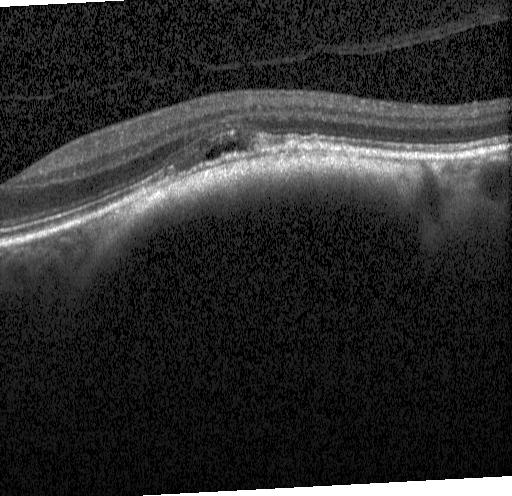

Spectral-domain optical coherence tomography; OCT B-scan; instrument: Heidelberg Spectralis; macular scan.
The scan shows choroidal neovascularization (CNV).